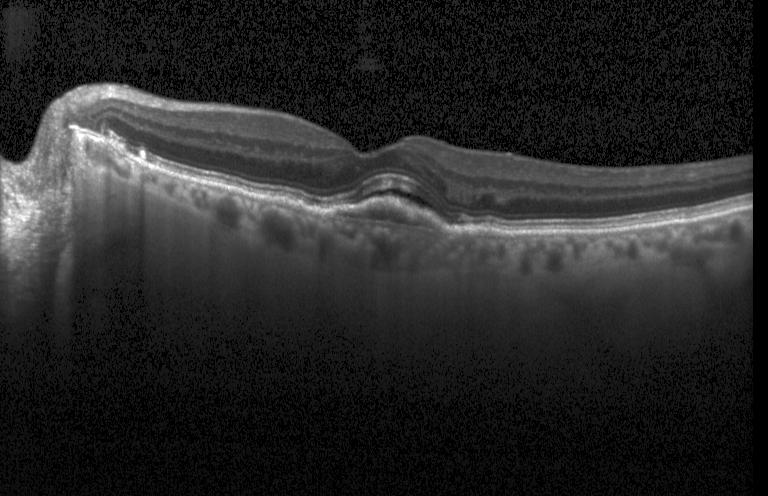 OCT line scan · SD-OCT · horizontal scan through the fovea. Finding: choroidal neovascularization (CNV).